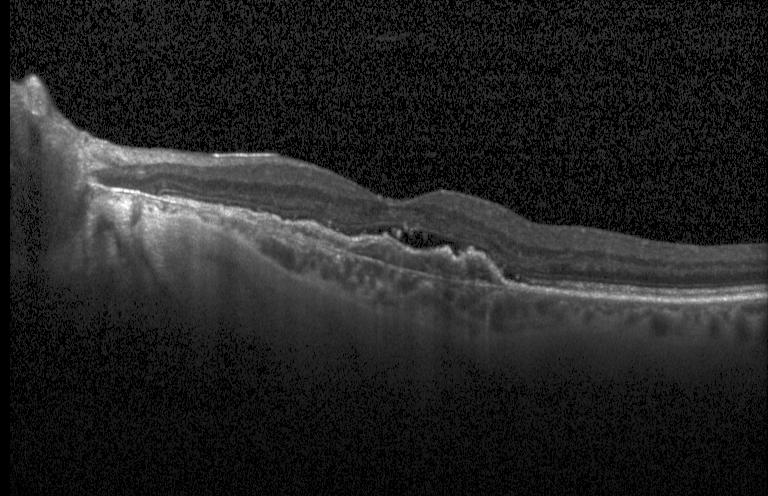

Optical coherence tomography B-scan.
Diagnosis: a choroidal neovascular membrane.